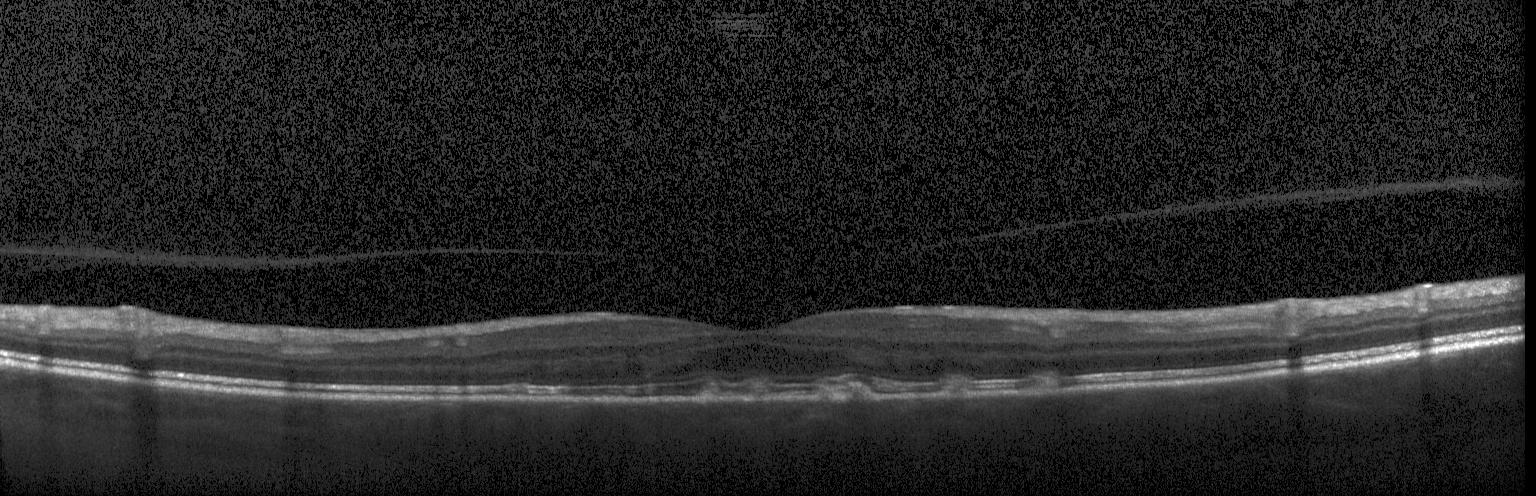

Multiple drusen.